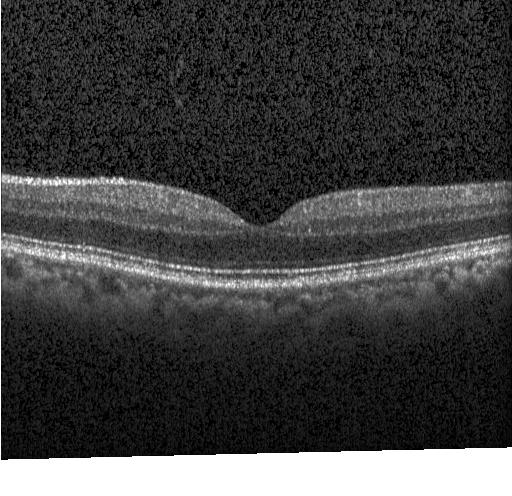

Optical coherence tomography B-scan; SD-OCT; Heidelberg Spectralis OCT system — Dx: no evidence of CNV, DME, or drusen.